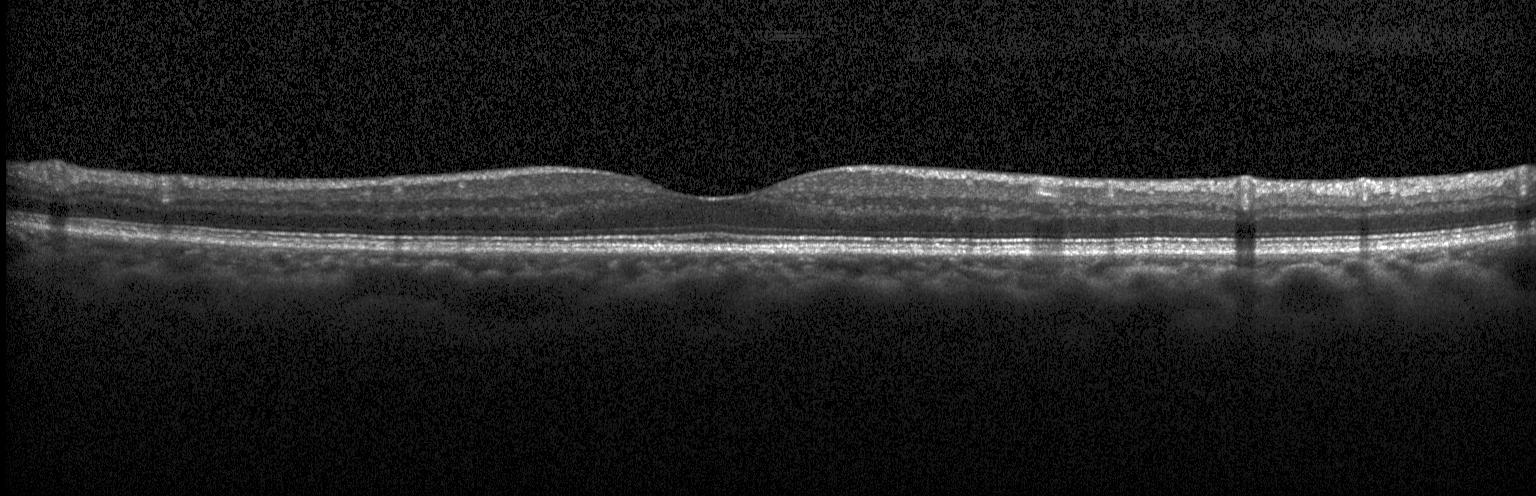 Macular OCT demonstrating no evidence of choroidal neovascularization, diabetic macular edema, or drusen.